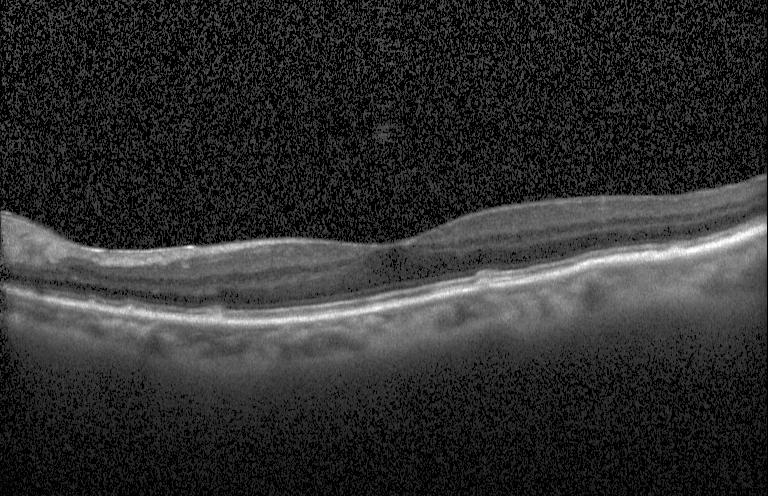
Acquired on a Heidelberg Spectralis; OCT B-scan.
This B-scan demonstrates drusen.